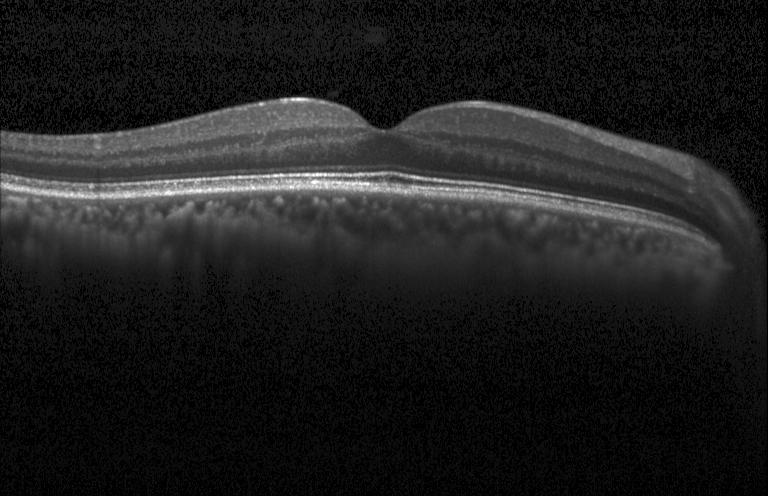
Diagnosis: no choroidal neovascularization, no diabetic macular edema, and no drusen.